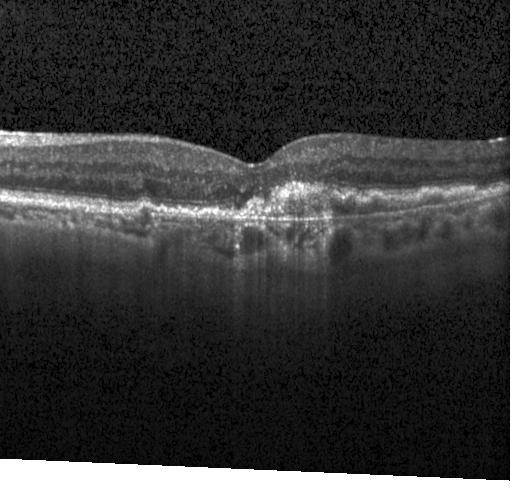

OCT line scan — Choroidal neovascularization (CNV).